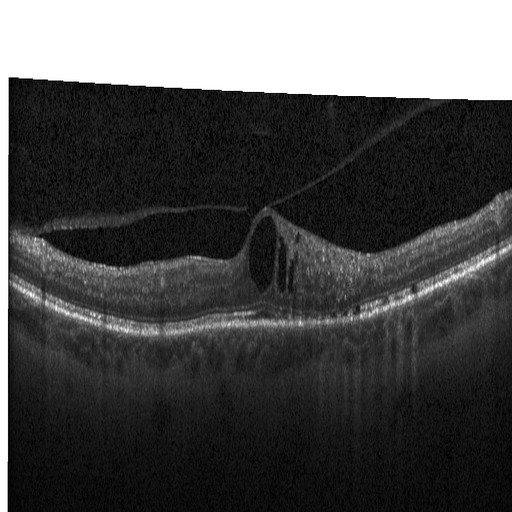

This B-scan demonstrates DME.